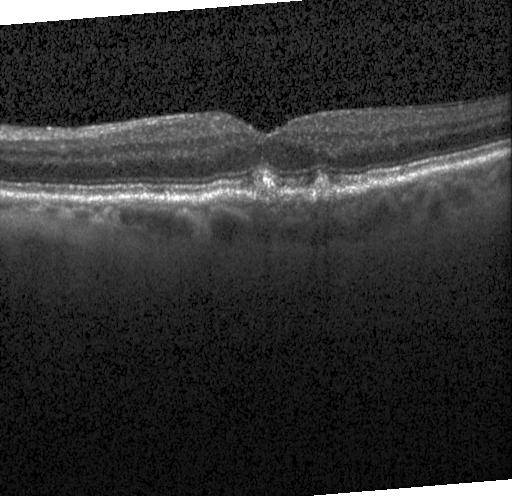

Optical coherence tomography scan. This B-scan demonstrates sub-RPE drusenoid deposits.